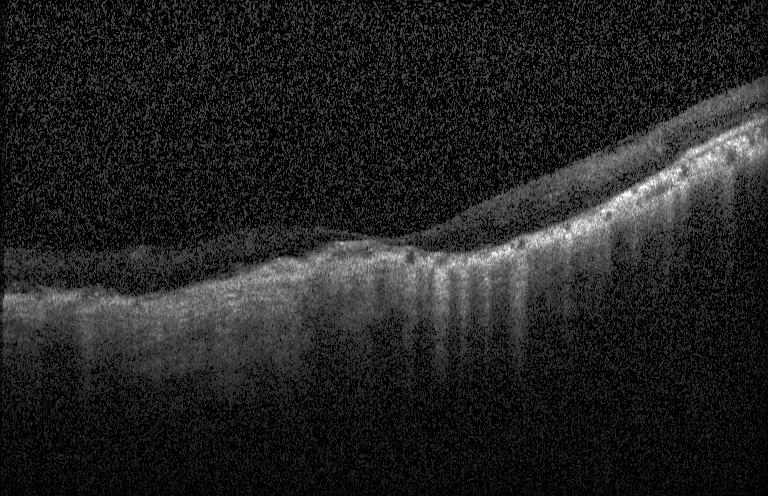 OCT B-scan; centered on the fovea; Heidelberg Spectralis OCT system
Macular OCT: a choroidal neovascular membrane.